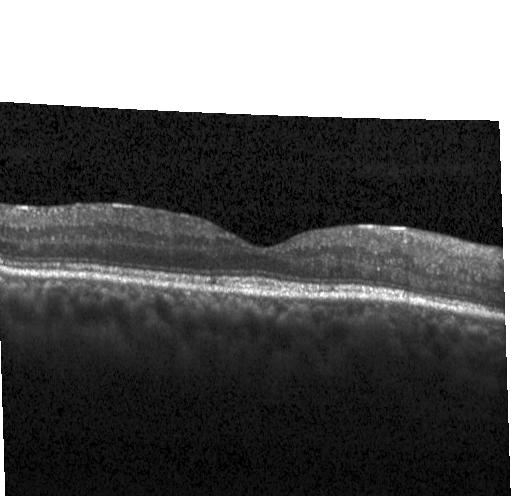
Retinal OCT cross-section showing no choroidal neovascularization, diabetic macular edema, or drusen.